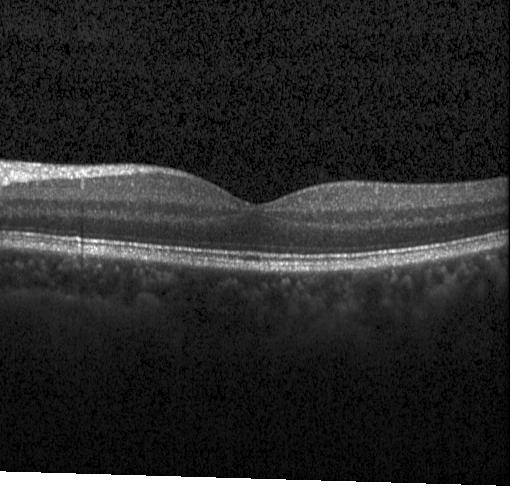
This B-scan demonstrates no evidence of choroidal neovascularization, diabetic macular edema, or drusen.